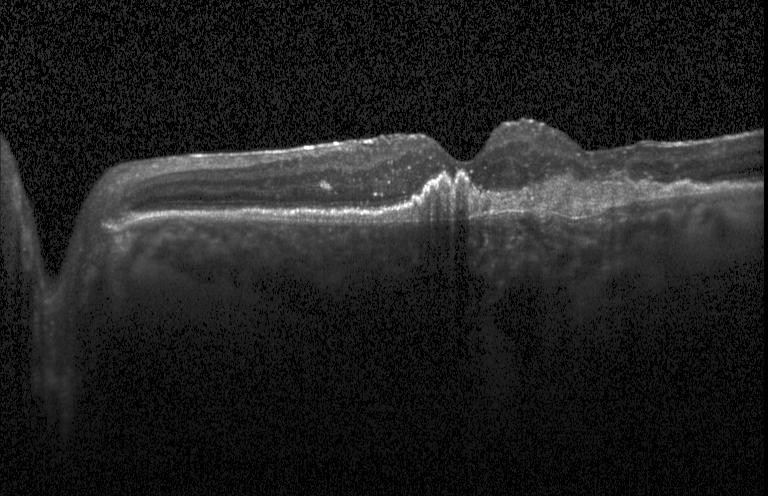

OCT B-scan.
CNV.